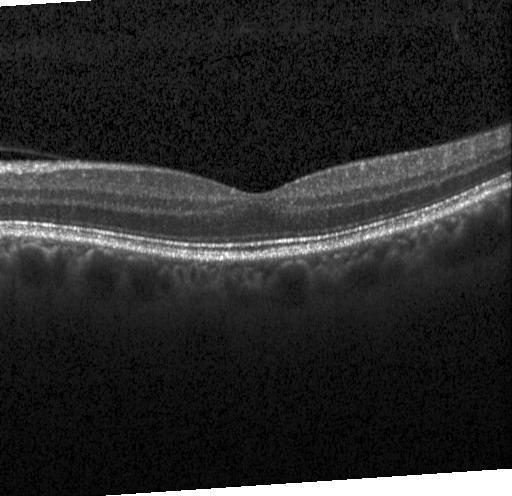

Optical coherence tomography B-scan
Finding: no evidence of choroidal neovascularization, diabetic macular edema, or drusen.